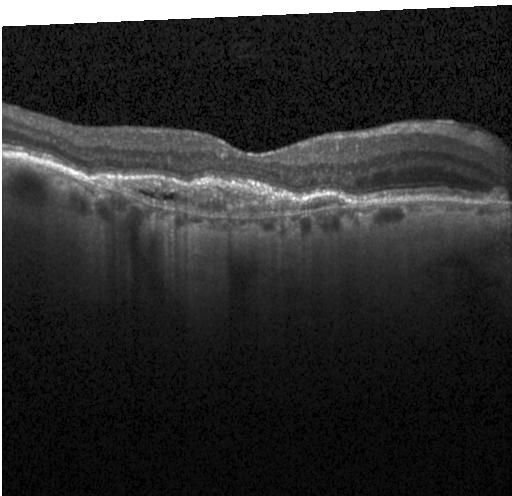
OCT finding: choroidal neovascularization.